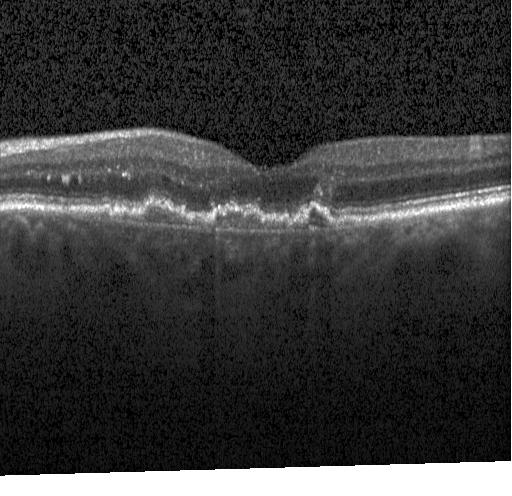
Spectral-domain OCT, Heidelberg Spectralis OCT system, fovea-centered, OCT B-scan.
This B-scan demonstrates a choroidal neovascular membrane.